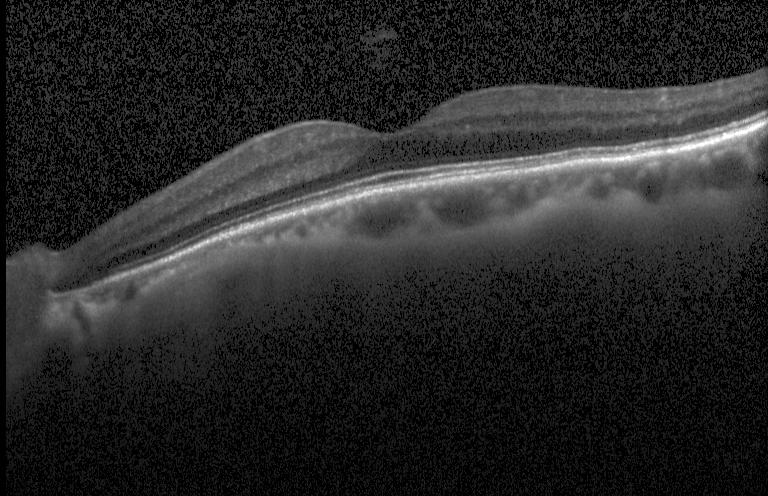
Heidelberg Spectralis OCT system; OCT line scan
Assessment: no evidence of CNV, DME, or drusen.